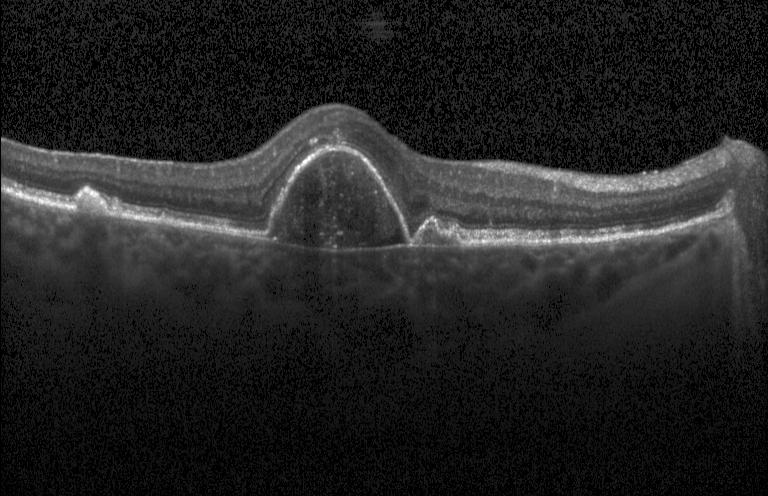

Choroidal neovascularization (CNV).